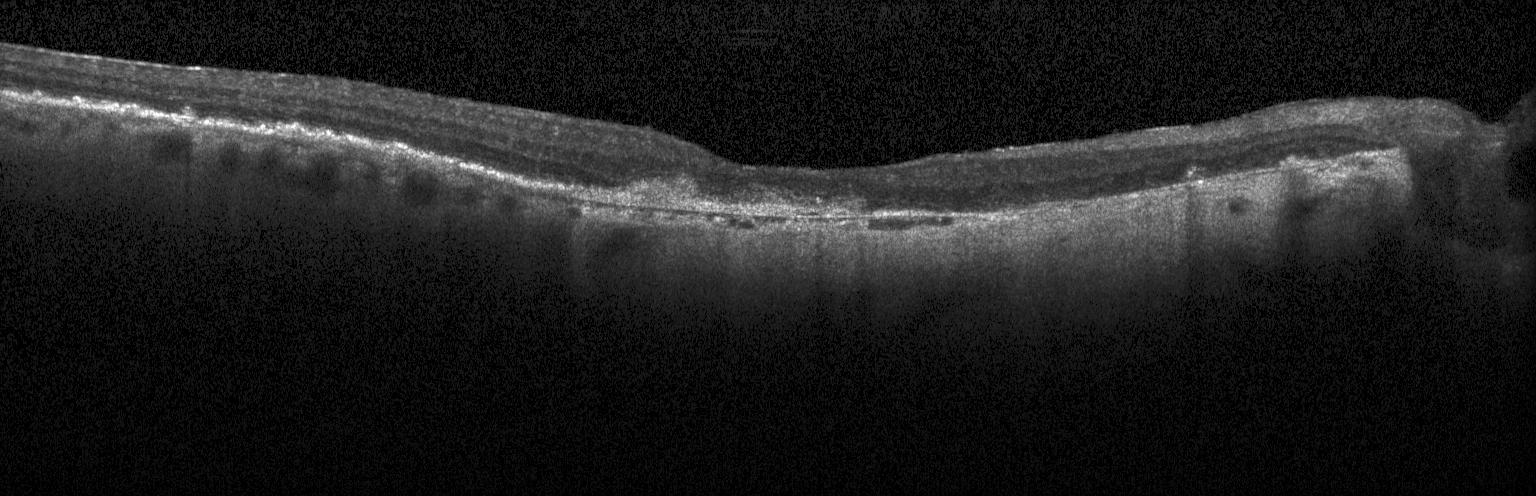

Diagnosis: choroidal neovascularization (CNV).